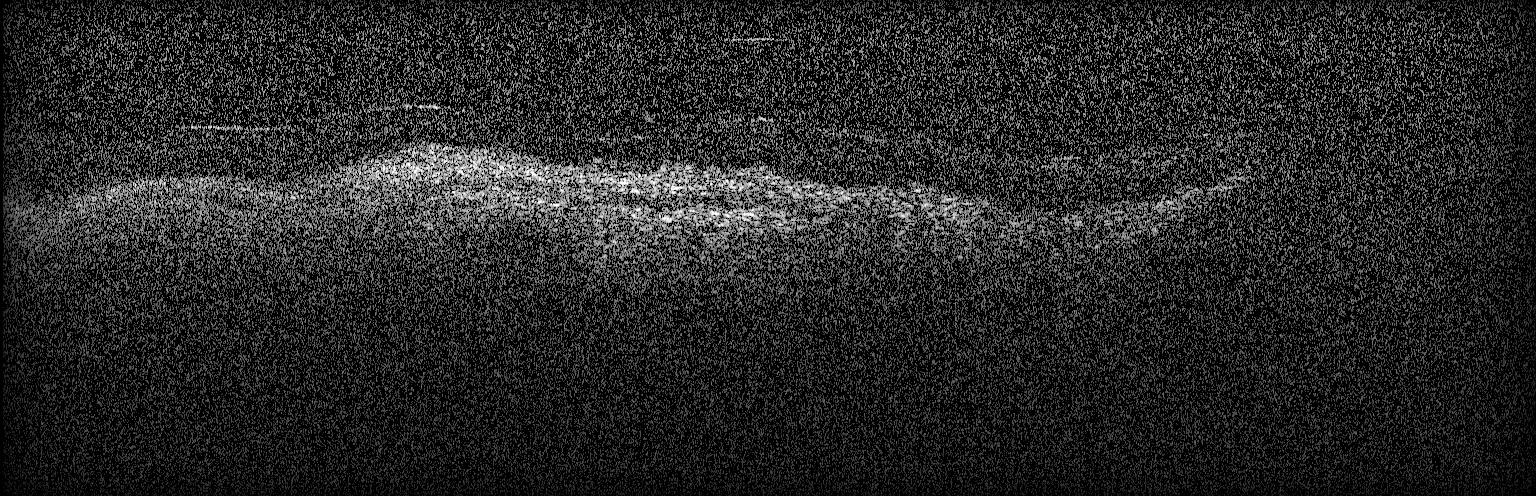
Impression: a choroidal neovascular membrane.